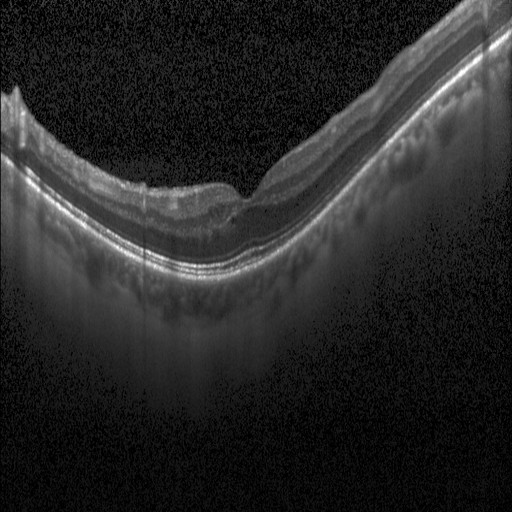 OCT B-scan — Impression: diabetic macular edema.